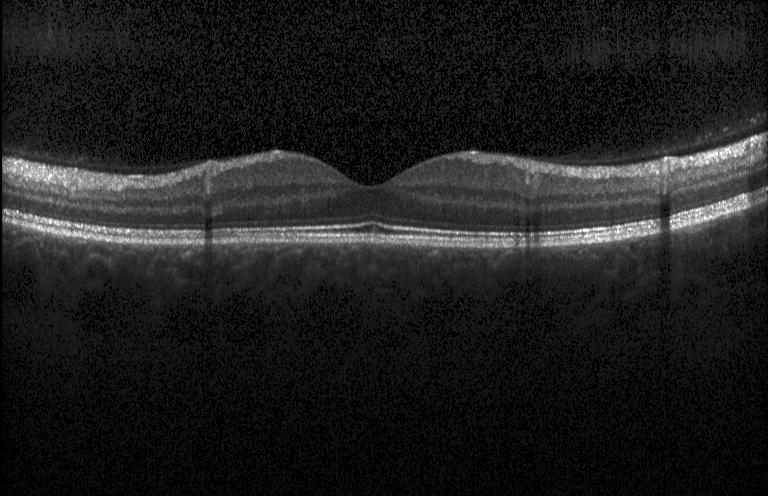

Centered on the fovea, OCT B-scan.
Impression: no choroidal neovascularization, diabetic macular edema, or drusen.